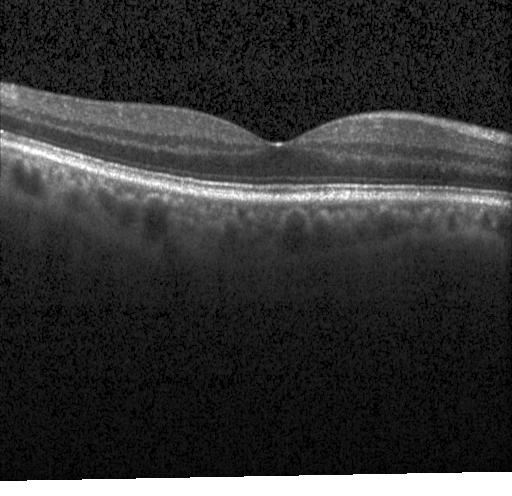
Diagnosis: no CNV, no DME, and no drusen.